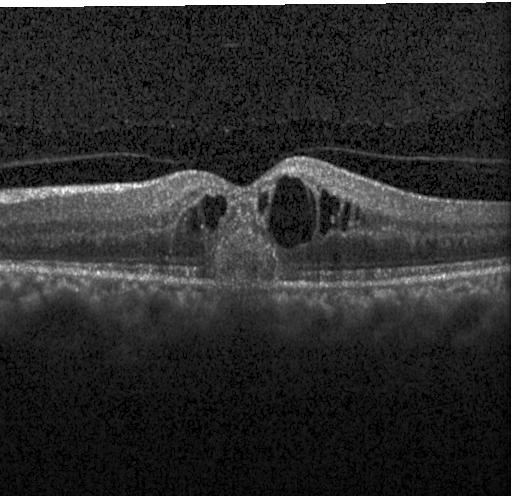 Retinal OCT cross-section, instrument: Heidelberg Spectralis
OCT finding: a choroidal neovascular membrane.